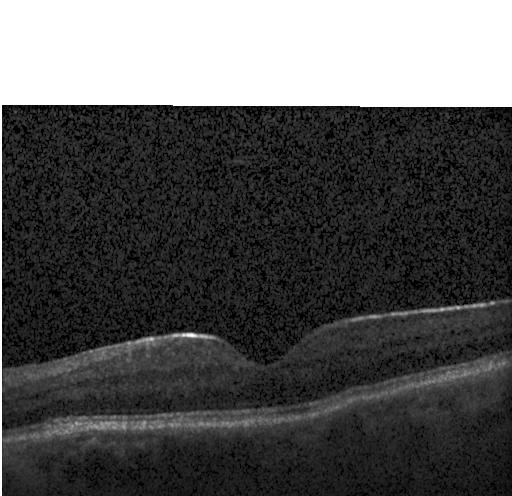 Impression: neither CNV, DME, nor drusen.